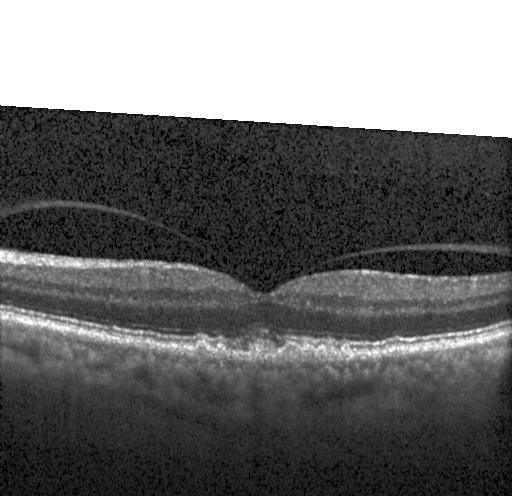 OCT B-scan. Instrument: Heidelberg Spectralis. Through the macula
Dx: drusen.